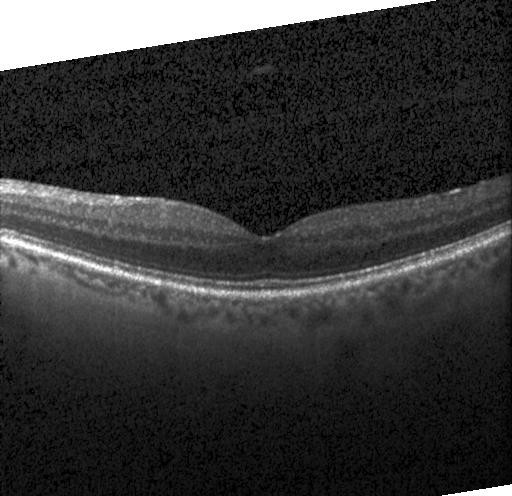
Finding: no evidence of choroidal neovascularization, diabetic macular edema, or drusen.